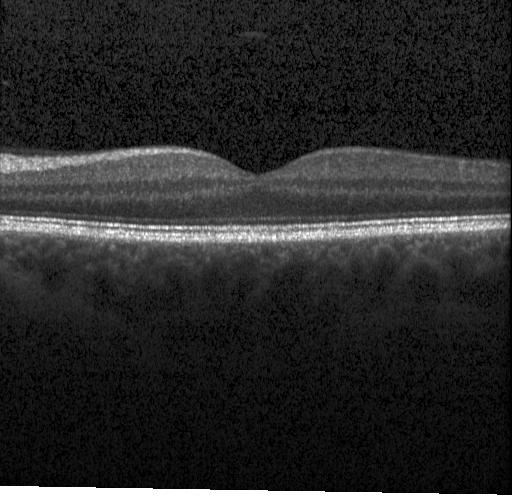 OCT finding: neither CNV, DME, nor drusen.